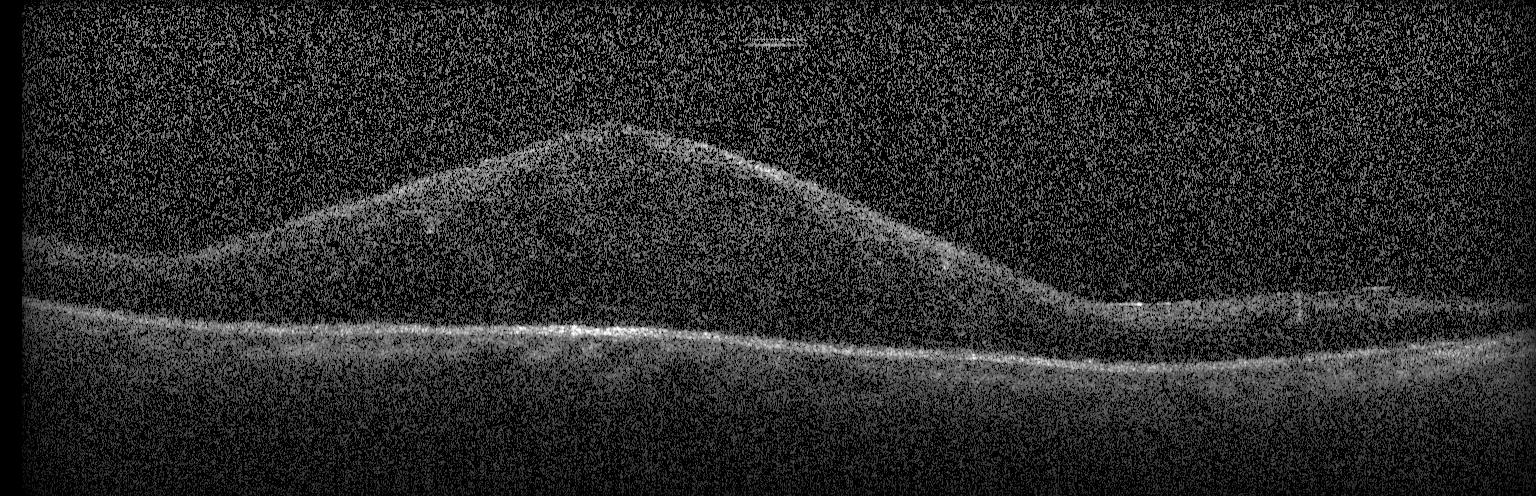
Retinal OCT B-scan.
This B-scan demonstrates diabetic macular edema.